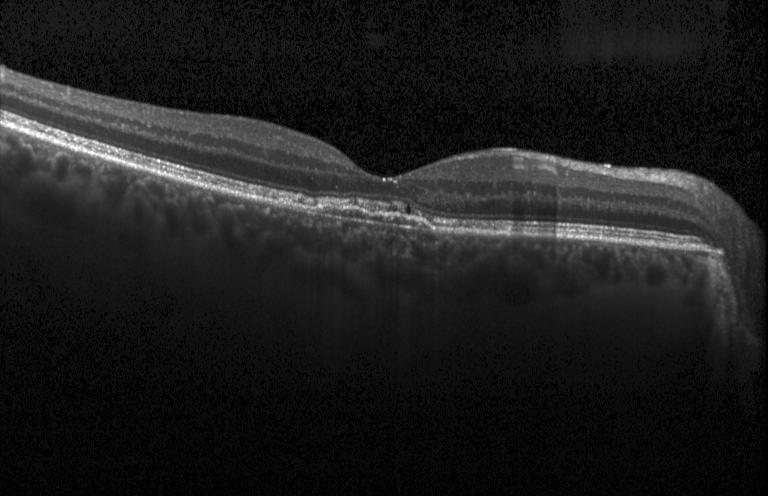

Horizontal scan through the fovea · SD-OCT · acquired on a Heidelberg Spectralis · OCT line scan.
The scan shows CNV.